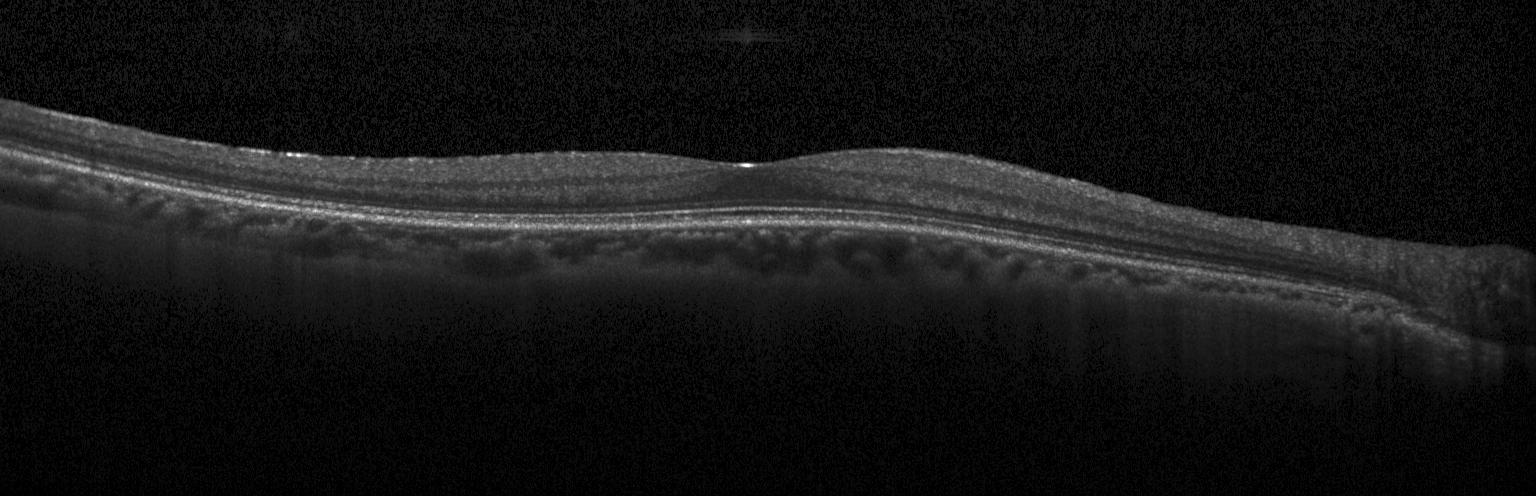 Assessment: no choroidal neovascularization, no diabetic macular edema, and no drusen.